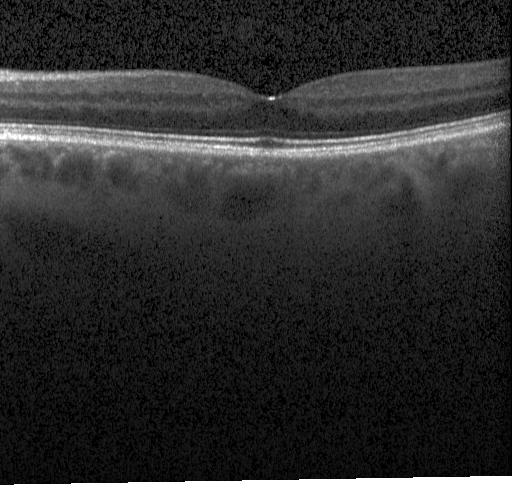 Fovea-centered. Heidelberg Spectralis. OCT line scan.
OCT finding: no choroidal neovascularization, no diabetic macular edema, and no drusen.